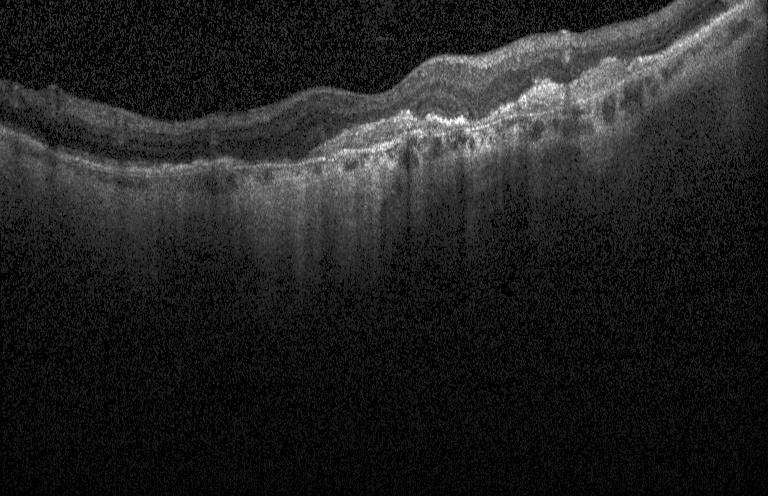 Spectral-domain OCT B-scan: a choroidal neovascular membrane.